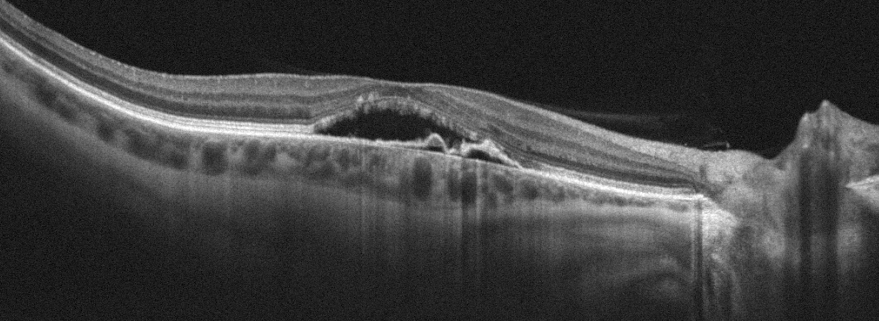 Retinal OCT cross-section. Dx: age-related macular degeneration (AMD).